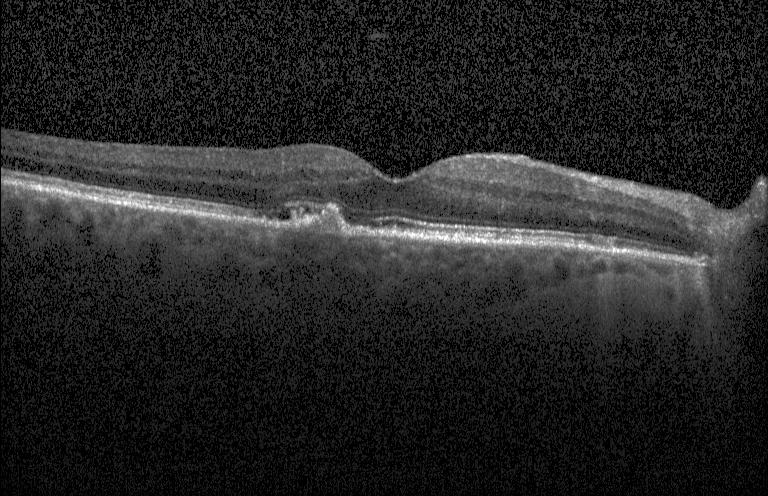 Spectral-domain OCT · Heidelberg Spectralis OCT system · OCT B-scan · centered on the fovea. The scan shows CNV.